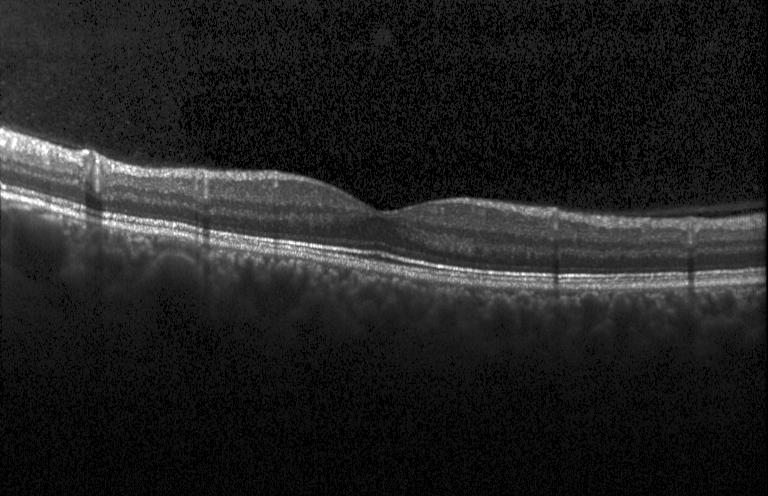
Optical coherence tomography B-scan. Fovea-centered.
Impression: no CNV, DME, or drusen.